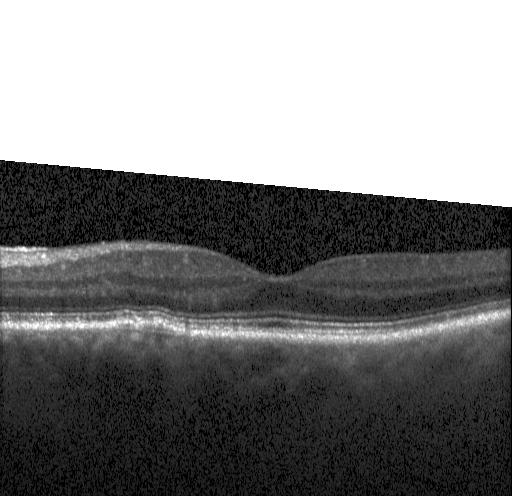
Impression: drusen.